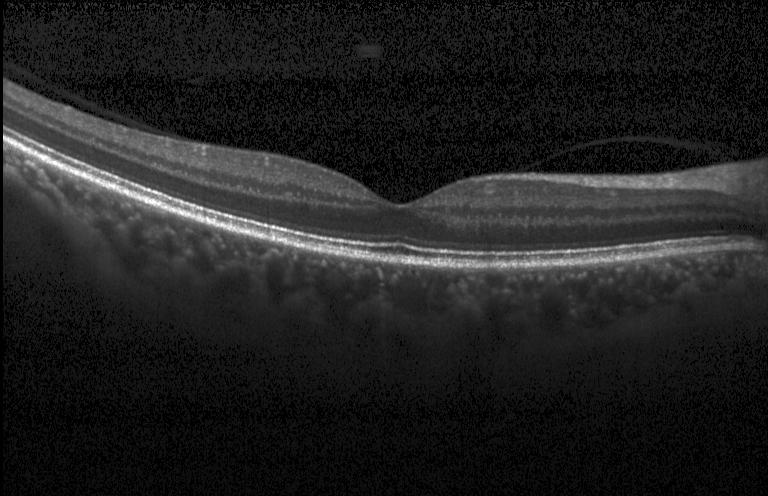 Spectral-domain OCT B-scan: no choroidal neovascularization, no diabetic macular edema, and no drusen.